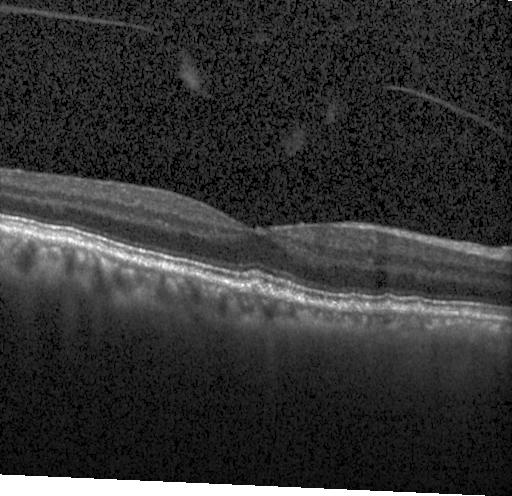
This B-scan demonstrates drusen.